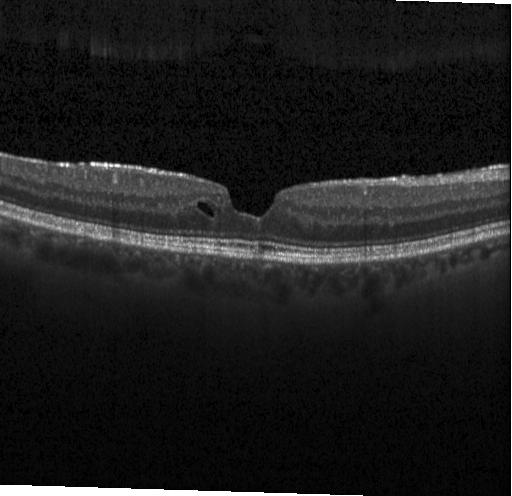

OCT B-scan showing diabetic macular edema (DME).